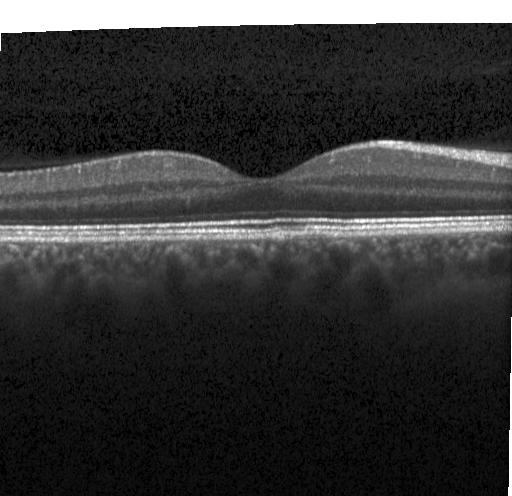
Diagnosis: no choroidal neovascularization, diabetic macular edema, or drusen.